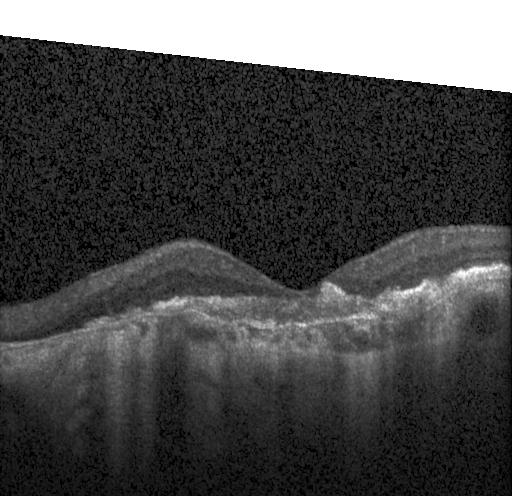
Optical coherence tomography scan.
This B-scan demonstrates a choroidal neovascular membrane.